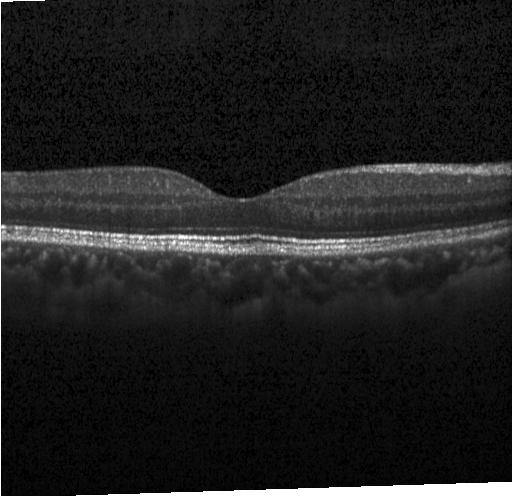
Finding: neither choroidal neovascularization, diabetic macular edema, nor drusen.